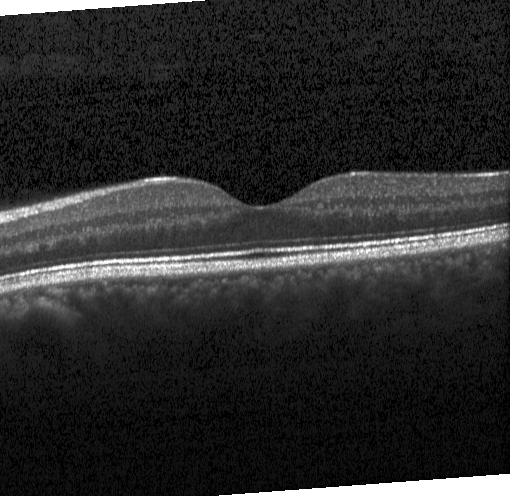 Spectral-domain OCT, OCT B-scan, through the macula, acquired on a Heidelberg Spectralis — Dx: neither choroidal neovascularization, diabetic macular edema, nor drusen.